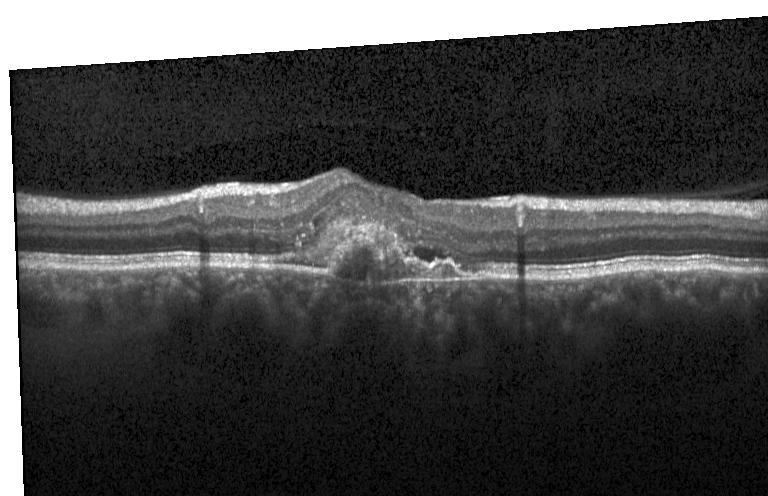 OCT finding: choroidal neovascularization (CNV).